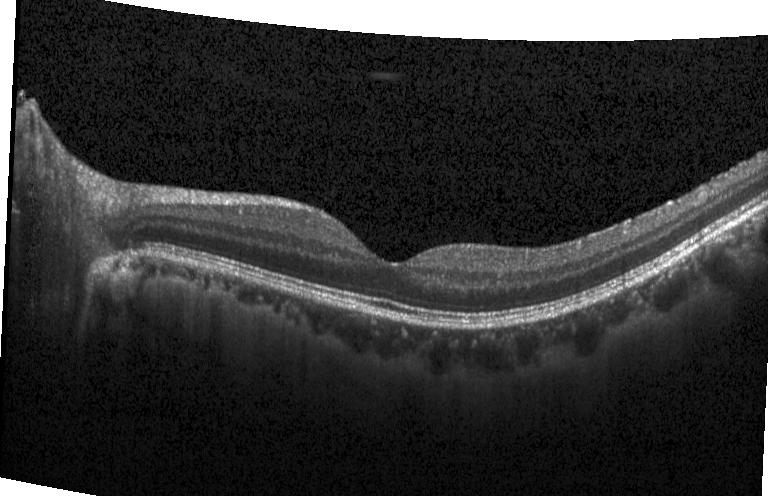

Horizontal scan through the fovea; optical coherence tomography scan; SD-OCT
Impression: no CNV, DME, or drusen.